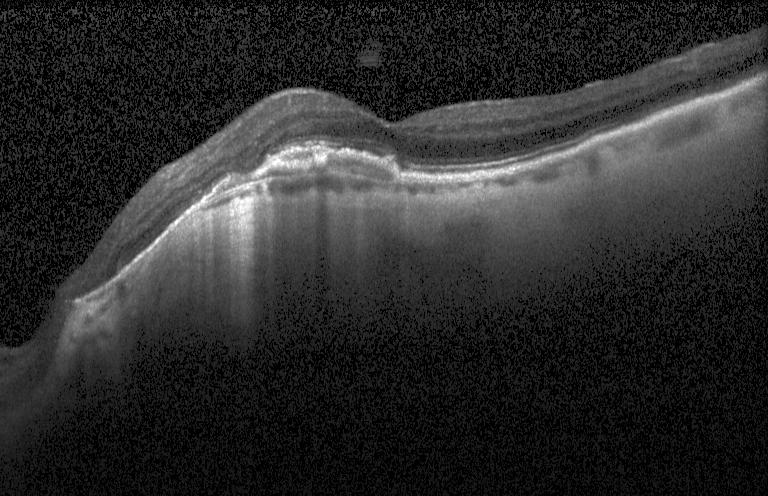

Centered on the fovea · retinal OCT B-scan · Heidelberg Spectralis.
Assessment: a choroidal neovascular membrane.